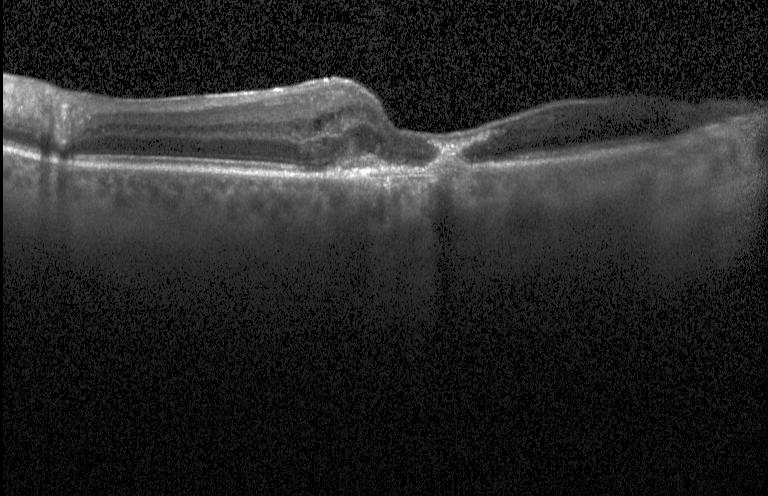

Through the macula. Acquired on a Heidelberg Spectralis. Retinal OCT cross-section
Dx: a choroidal neovascular membrane.